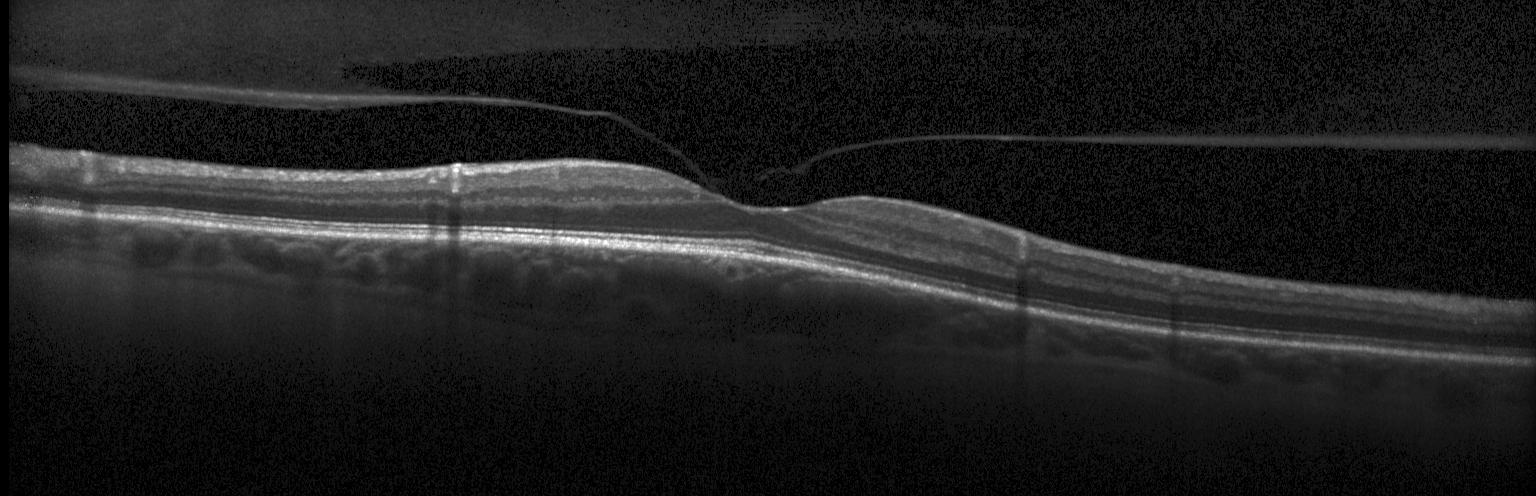

Impression: no evidence of CNV, DME, or drusen.